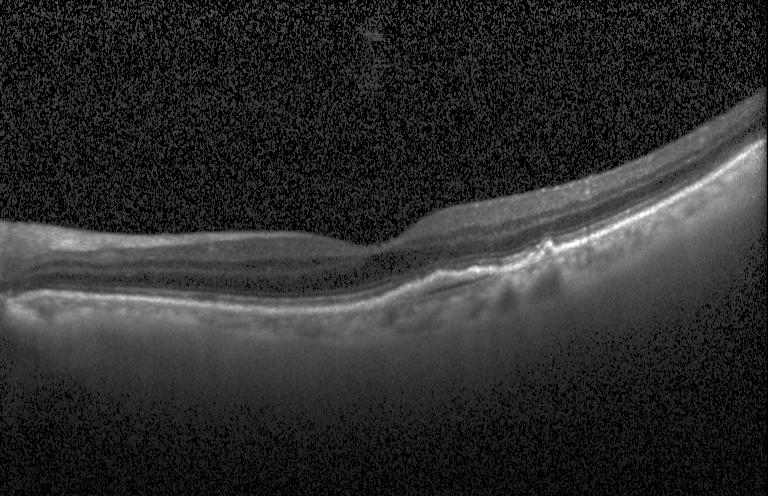
This B-scan demonstrates choroidal neovascularization (CNV).